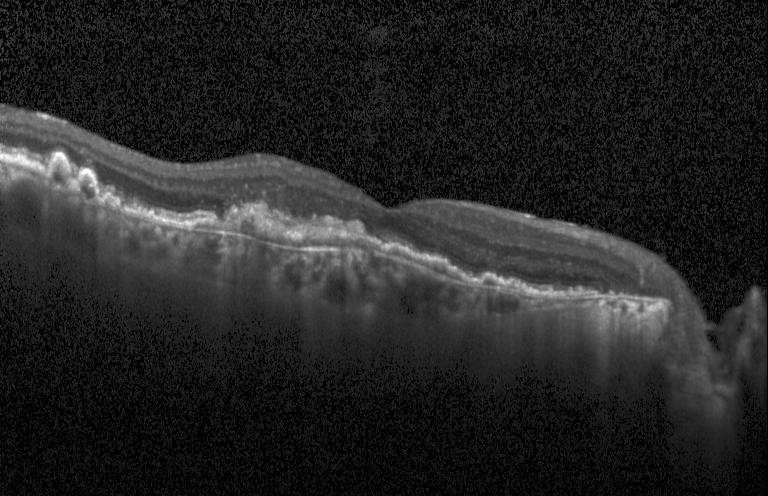 OCT finding: CNV.